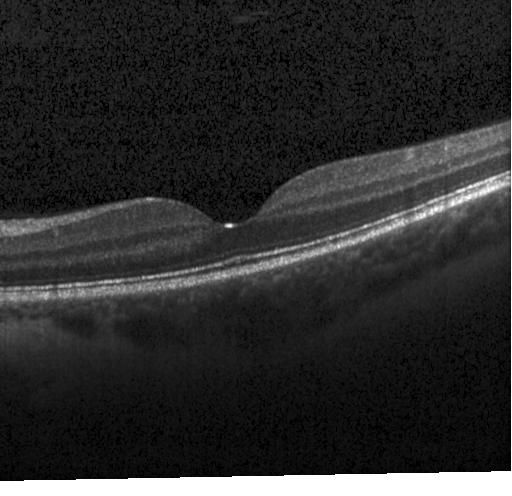

Optical coherence tomography scan
Impression: no CNV, no DME, and no drusen.